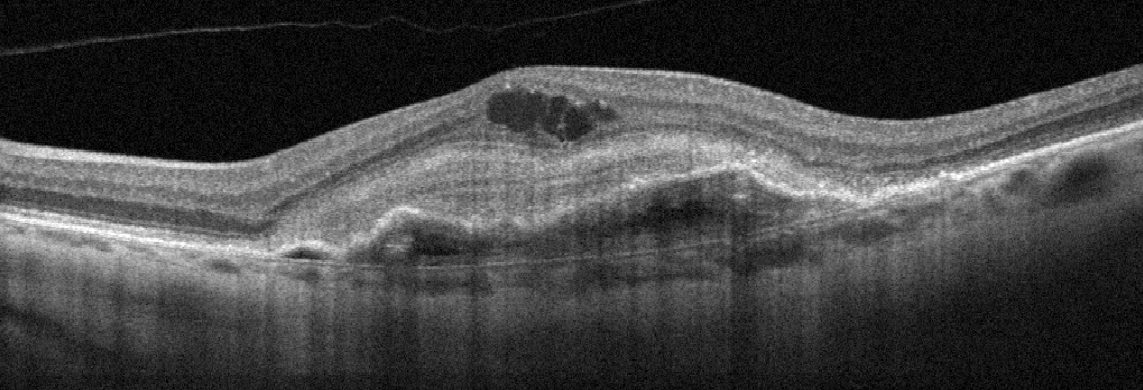 Optical coherence tomography B-scan. Through the macula. Instrument: Optovue Avanti RTVue XR. Impression: age-related macular degeneration (AMD).